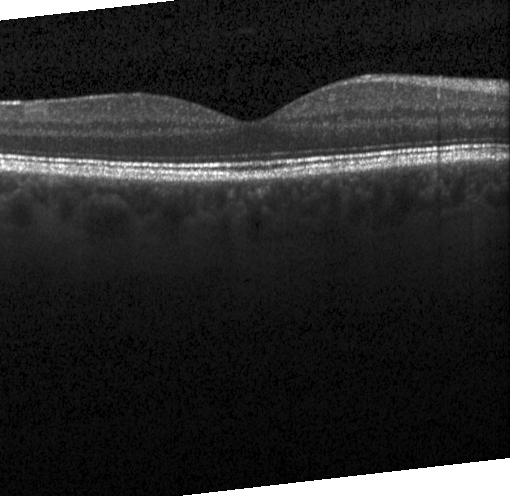
OCT B-scan. Diagnosis: no choroidal neovascularization, no diabetic macular edema, and no drusen.